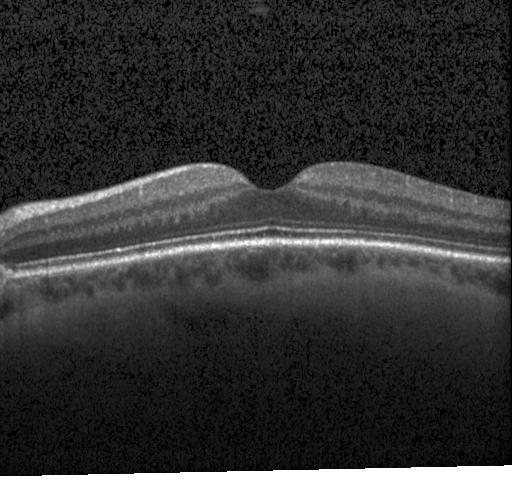 OCT finding: no CNV, DME, or drusen.